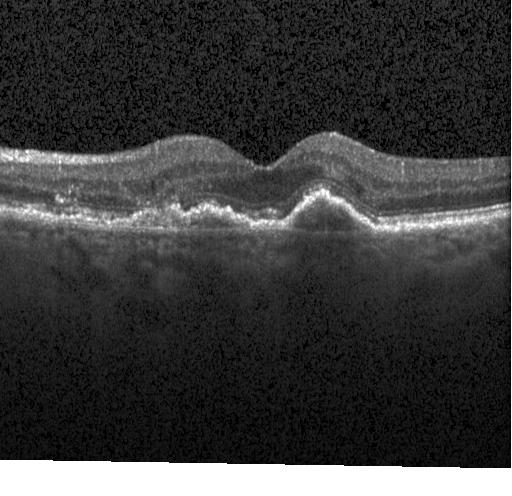 OCT scan showing a choroidal neovascular membrane.